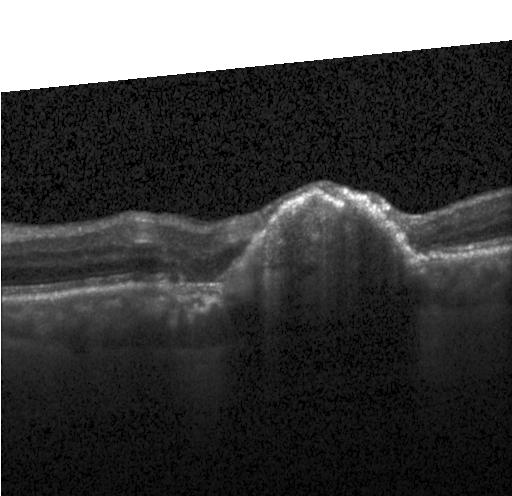 Spectral-domain OCT B-scan: choroidal neovascularization (CNV).